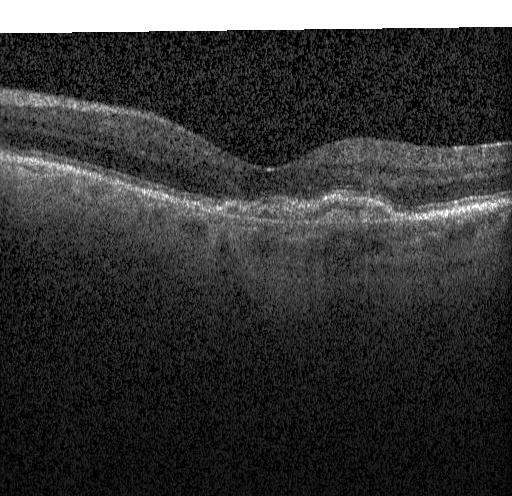
Assessment: a choroidal neovascular membrane.